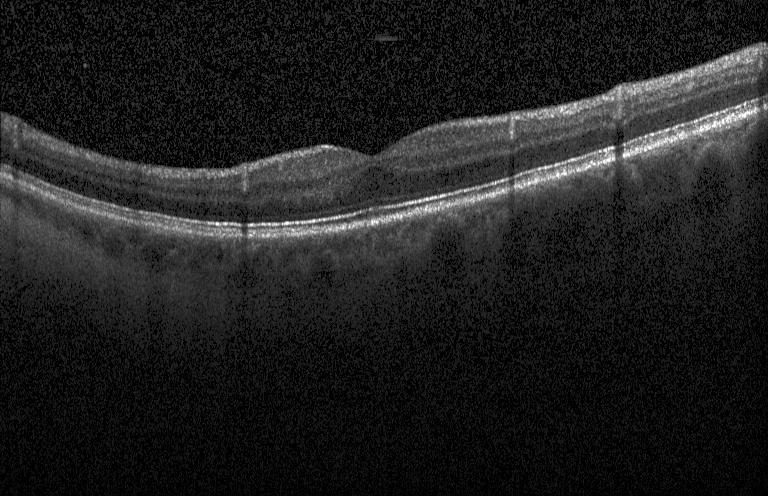 Spectral-domain OCT. Retinal OCT B-scan
Diagnosis: no choroidal neovascularization, diabetic macular edema, or drusen.